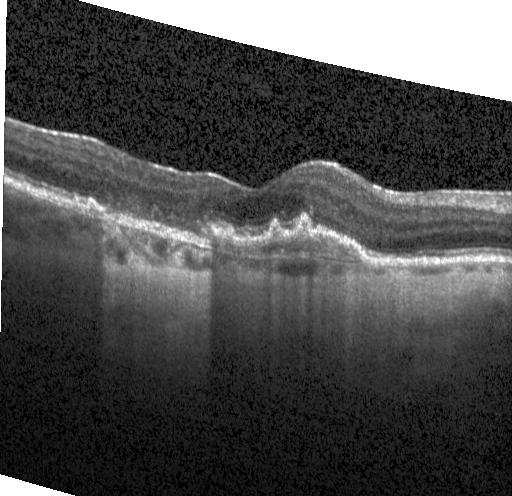

OCT B-scan — Dx: a choroidal neovascular membrane.